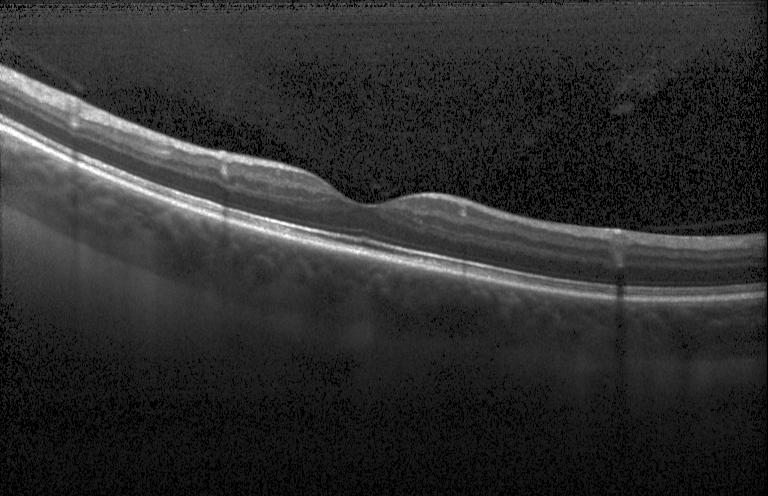

Diagnosis: no evidence of choroidal neovascularization, diabetic macular edema, or drusen.